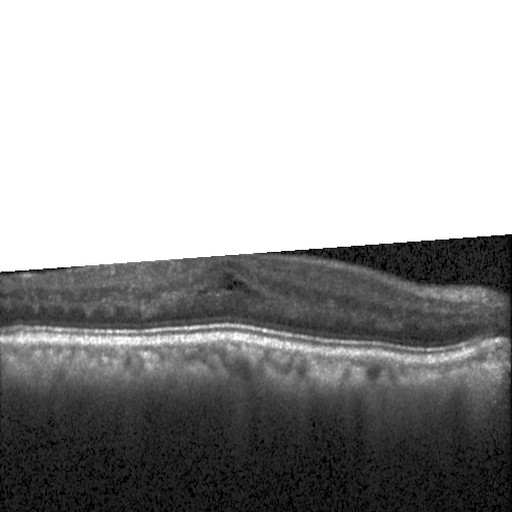 SD-OCT, Heidelberg Spectralis, fovea-centered, OCT line scan.
Impression: diabetic macular edema (DME).